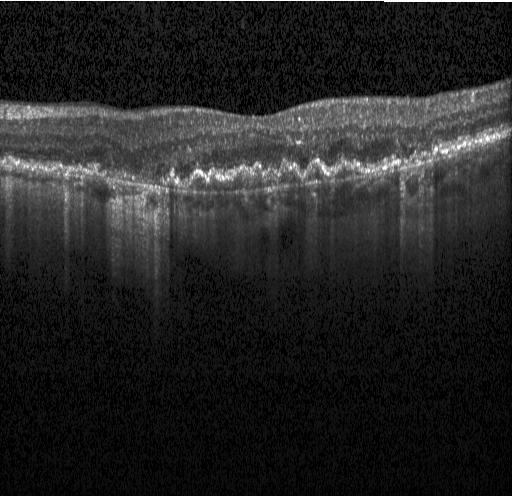 Finding: a choroidal neovascular membrane.